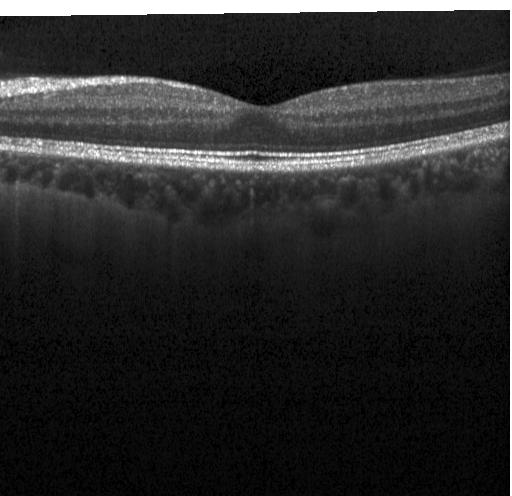

OCT B-scan showing neither choroidal neovascularization, diabetic macular edema, nor drusen.